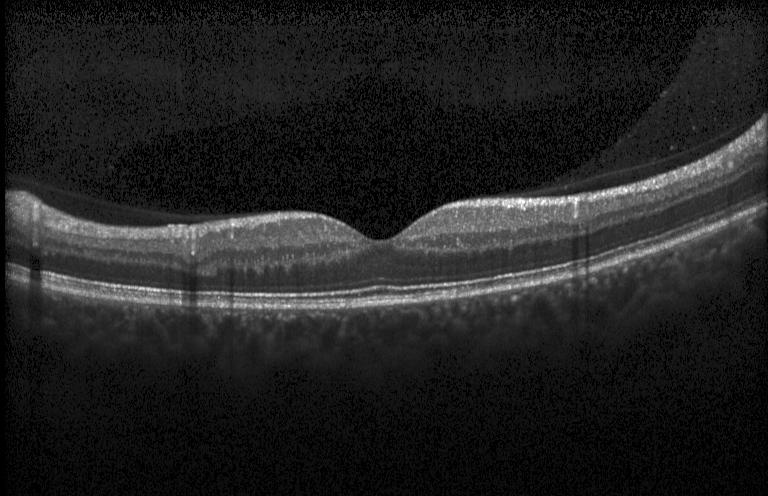
Acquired on a Heidelberg Spectralis. OCT B-scan. Fovea-centered
Impression: no evidence of CNV, DME, or drusen.